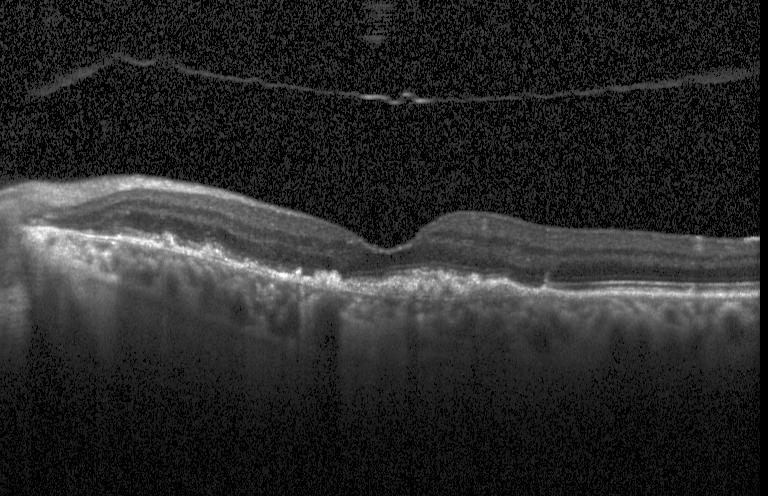 Acquired on a Heidelberg Spectralis; retinal OCT B-scan; spectral-domain optical coherence tomography — Diagnosis: a choroidal neovascular membrane.